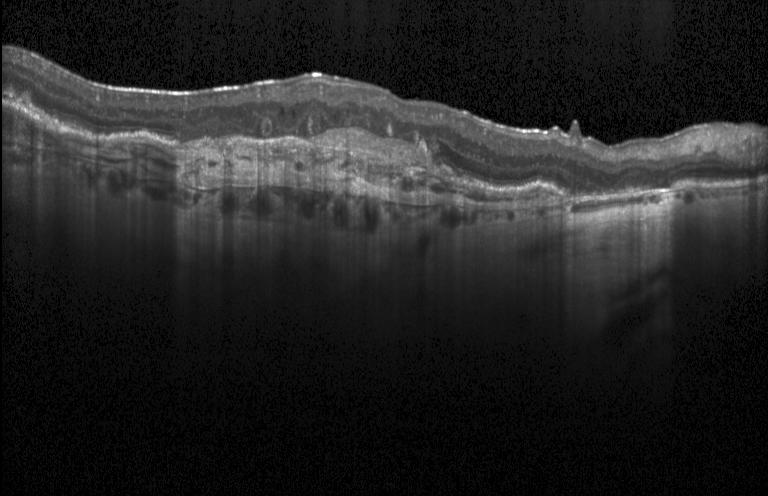 Acquired on a Heidelberg Spectralis. Spectral-domain OCT. Optical coherence tomography B-scan. Centered on the fovea — Diagnosis: a choroidal neovascular membrane.